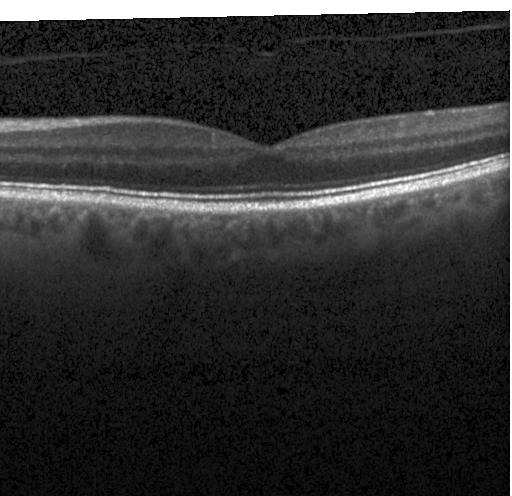
Spectral-domain OCT · optical coherence tomography B-scan.
Impression: neither CNV, DME, nor drusen.